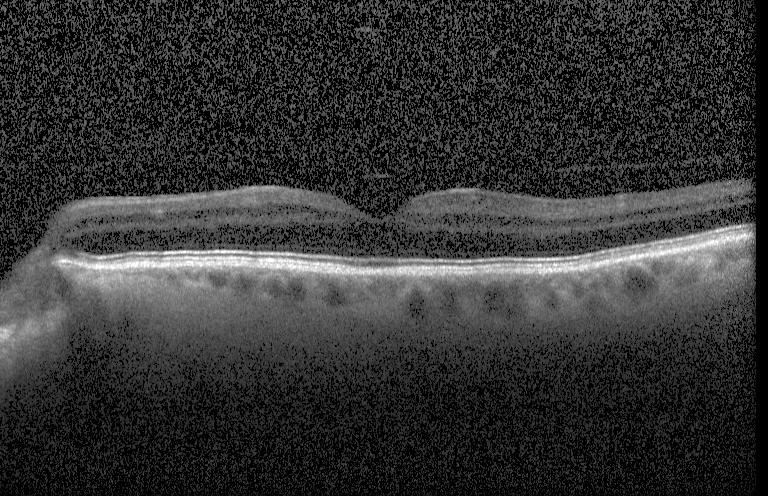

OCT B-scan, spectral-domain optical coherence tomography, acquired on a Heidelberg Spectralis, fovea-centered.
The scan shows no CNV, DME, or drusen.